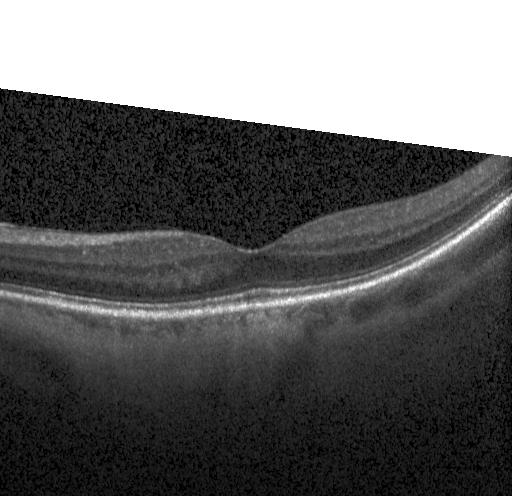

OCT finding: no CNV, no DME, and no drusen.